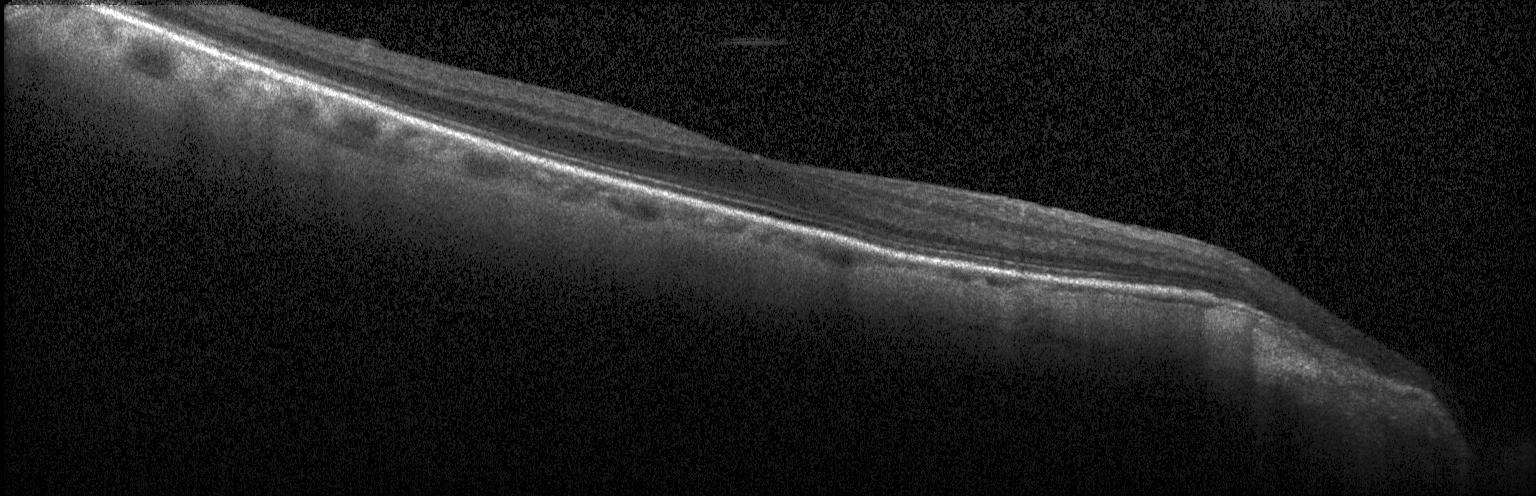
OCT B-scan.
OCT finding: no evidence of choroidal neovascularization, diabetic macular edema, or drusen.